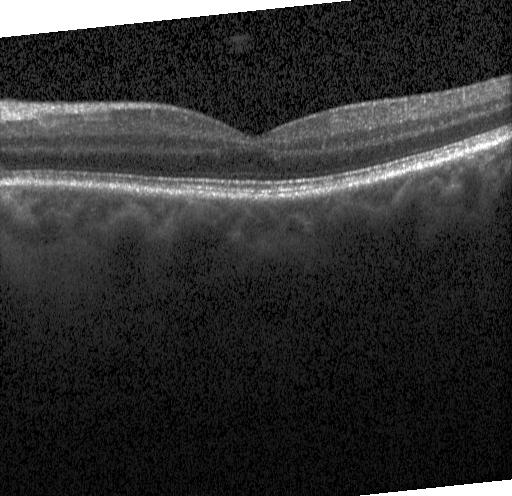

Optical coherence tomography B-scan
The scan shows no choroidal neovascularization, diabetic macular edema, or drusen.